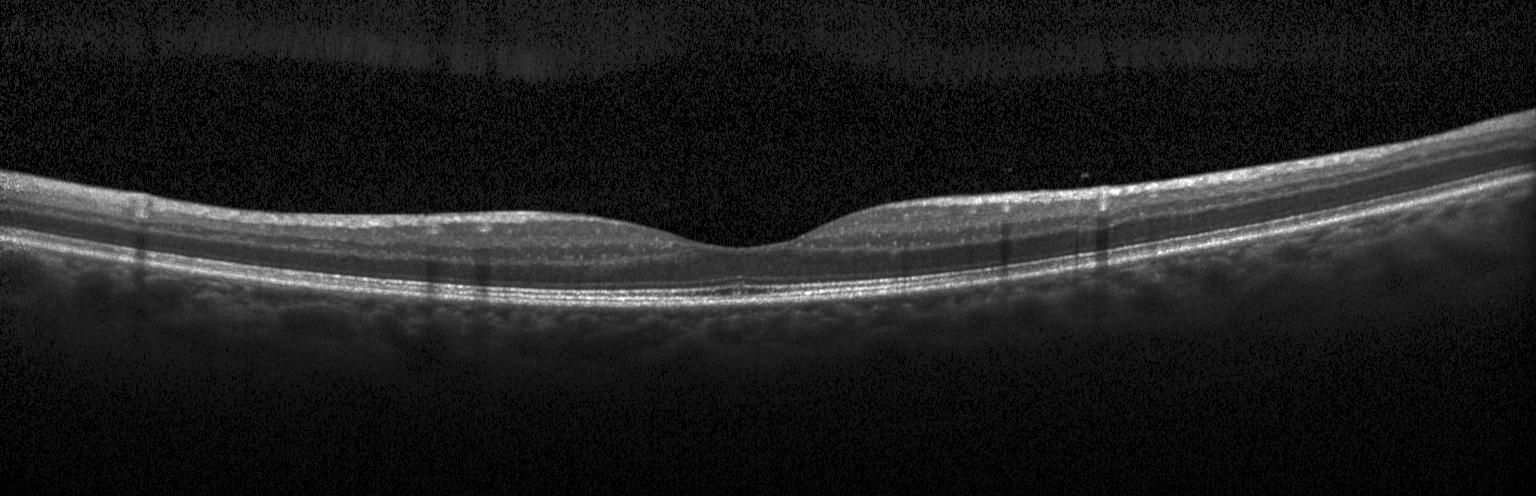
Optical coherence tomography B-scan; spectral-domain OCT; Heidelberg Spectralis OCT system. The scan shows neither choroidal neovascularization, diabetic macular edema, nor drusen.